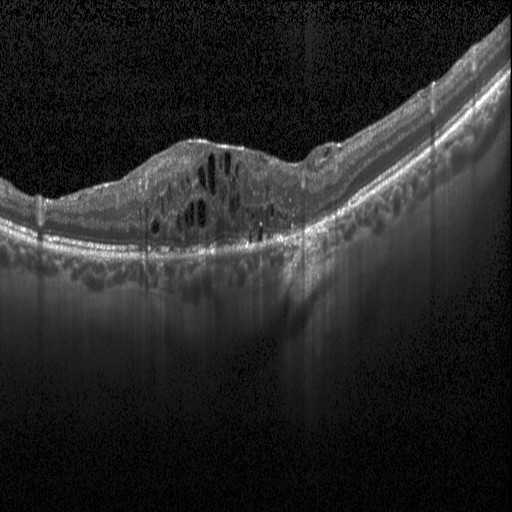

Retinal OCT cross-section — Finding: DME.